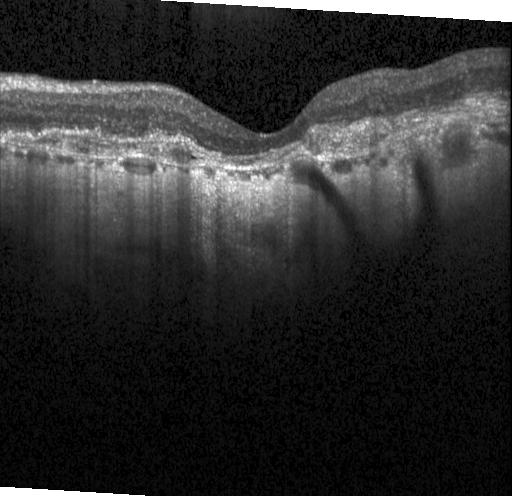 SD-OCT. Retinal OCT B-scan — Finding: a choroidal neovascular membrane.